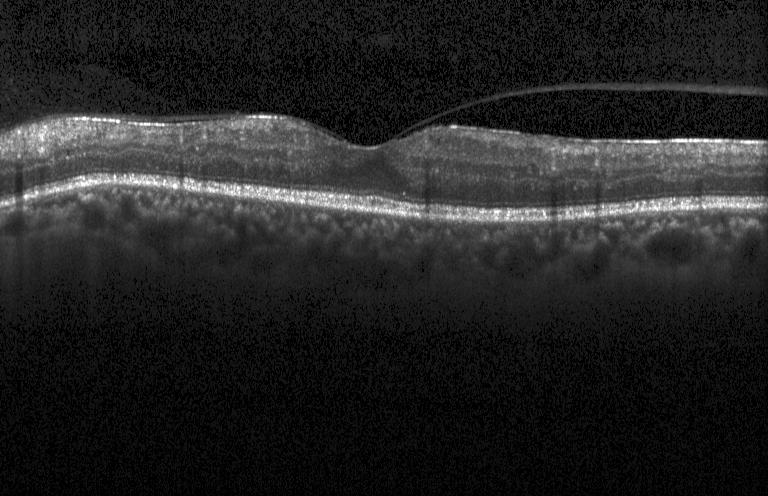

Optical coherence tomography scan
The scan shows diabetic macular edema.